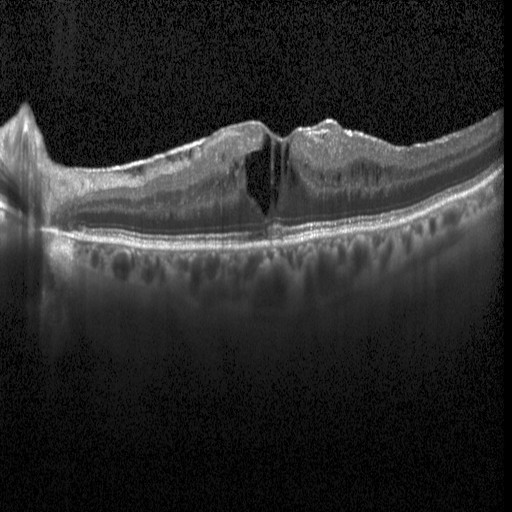

Retinal OCT B-scan. Dx: diabetic macular edema (DME).